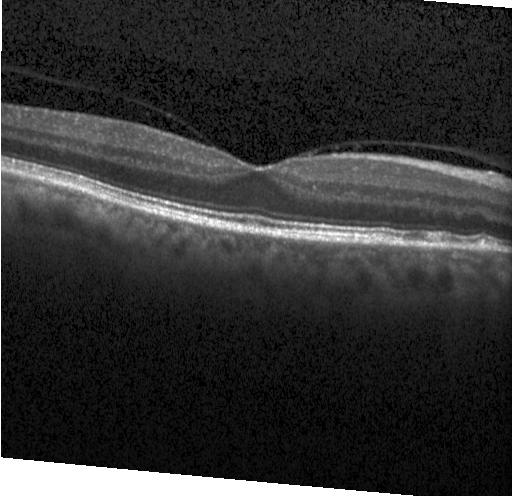 OCT B-scan showing drusen.